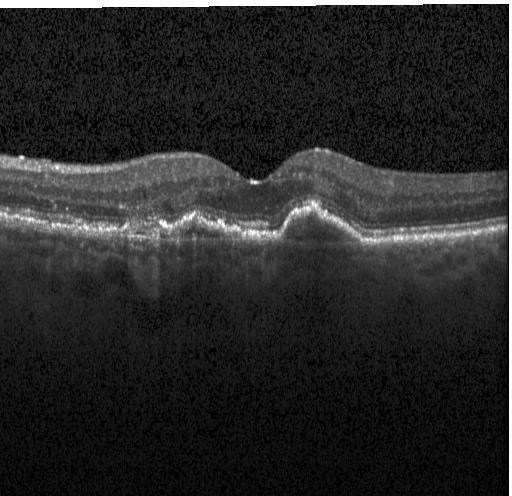 Choroidal neovascularization.